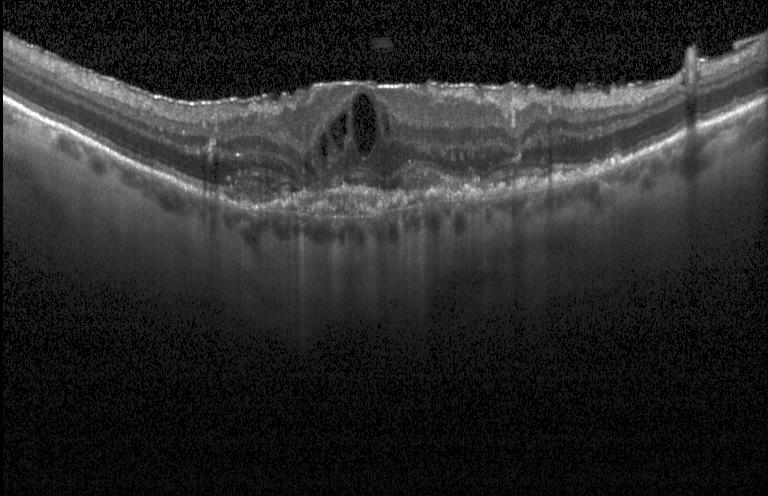
Diagnosis: a choroidal neovascular membrane.